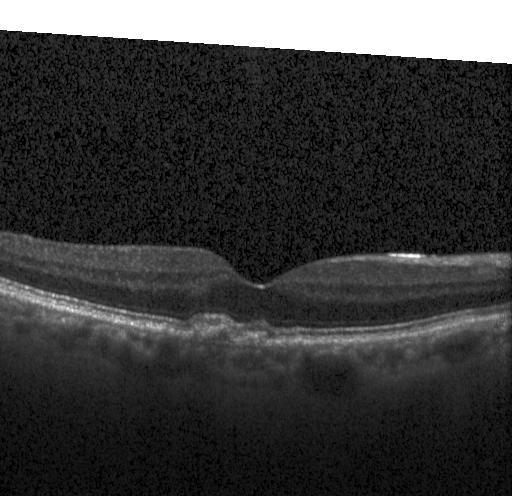

Dx: a choroidal neovascular membrane.